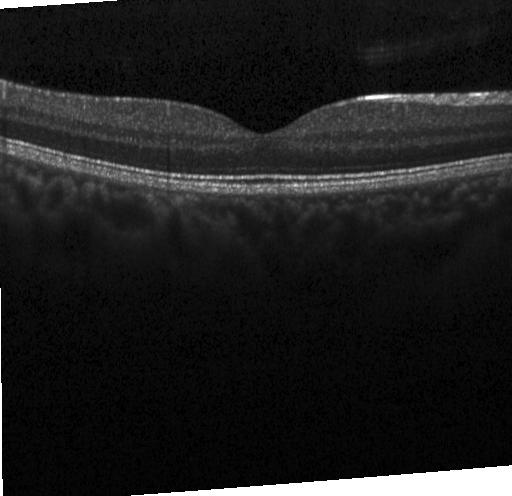

Retinal OCT cross-section.
This B-scan demonstrates neither choroidal neovascularization, diabetic macular edema, nor drusen.